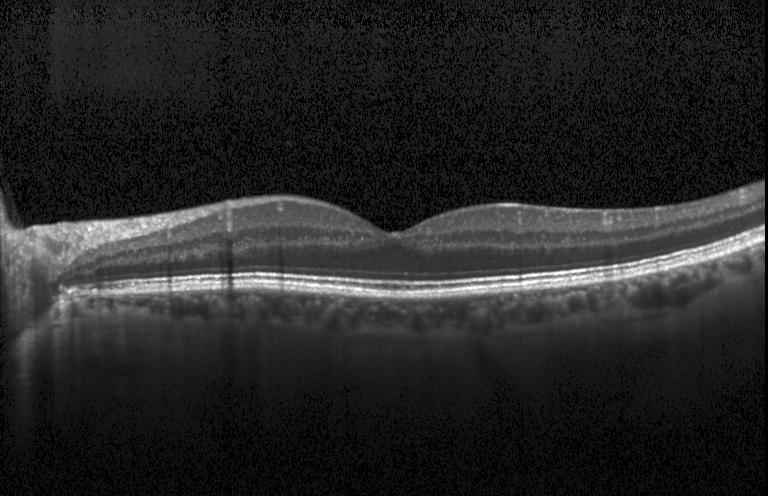
Centered on the fovea; spectral-domain optical coherence tomography; retinal OCT cross-section; Heidelberg Spectralis — Impression: no evidence of choroidal neovascularization, diabetic macular edema, or drusen.